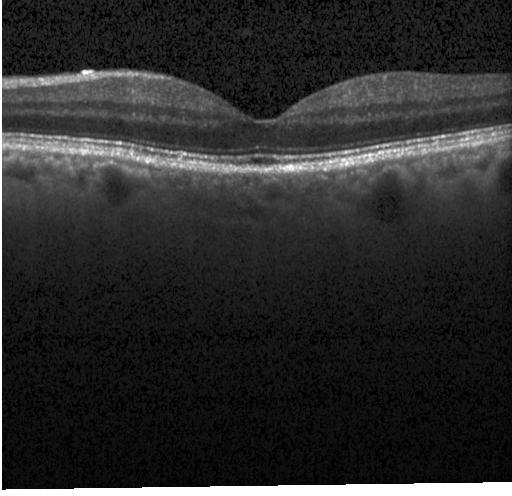

Optical coherence tomography scan; Heidelberg Spectralis; centered on the fovea; SD-OCT
Diagnosis: no choroidal neovascularization, no diabetic macular edema, and no drusen.